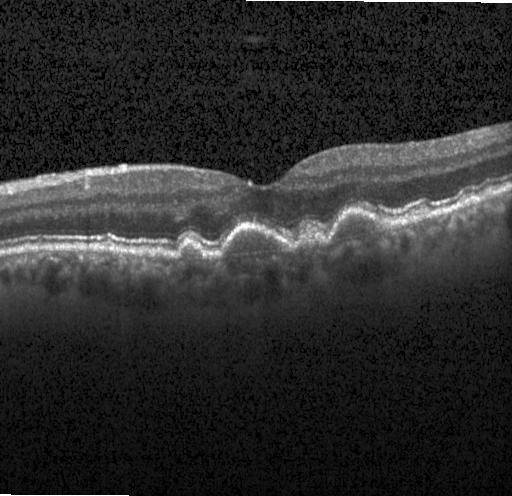 Optical coherence tomography B-scan · centered on the fovea · instrument: Heidelberg Spectralis · SD-OCT
OCT finding: drusen.